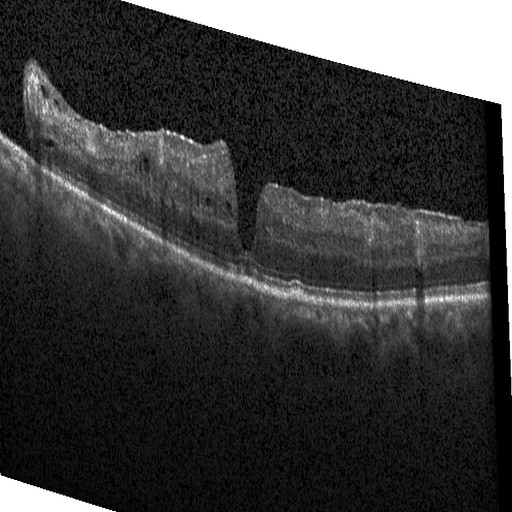
Centered on the fovea, optical coherence tomography B-scan
The scan shows DME.